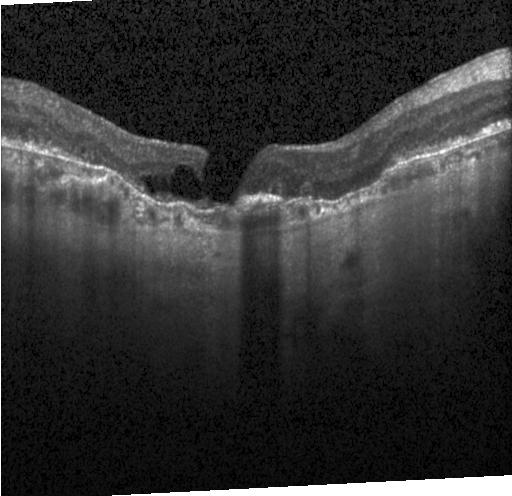 Centered on the fovea, OCT B-scan. Assessment: choroidal neovascularization (CNV).